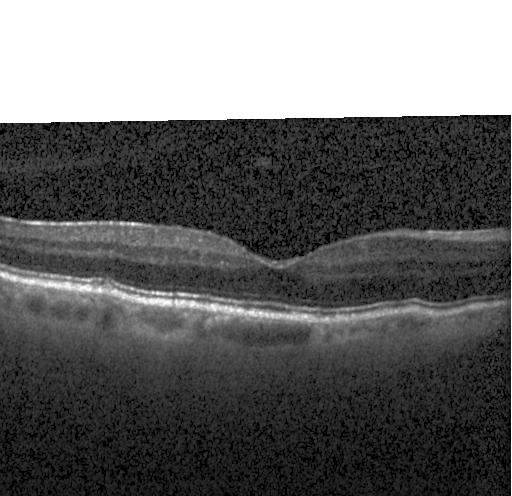
Impression: neither CNV, DME, nor drusen.